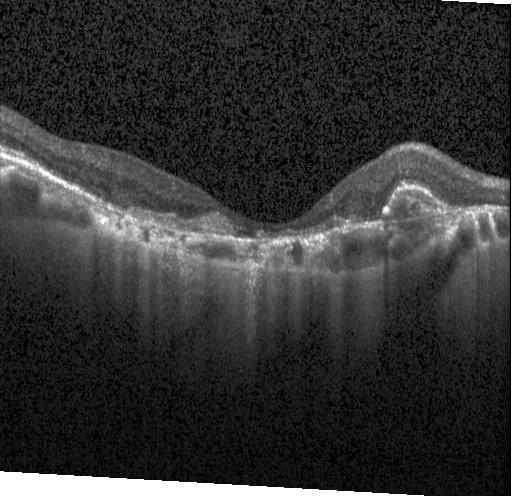

Through the macula, retinal OCT B-scan
Diagnosis: a choroidal neovascular membrane.